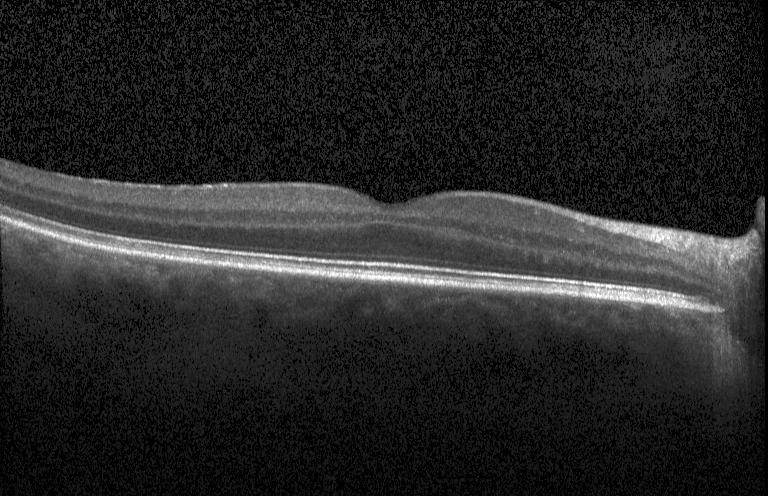

Spectral-domain optical coherence tomography; through the macula; optical coherence tomography scan.
No CNV, DME, or drusen.